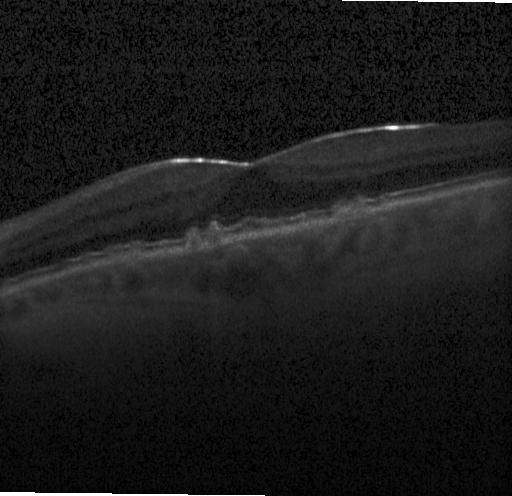

OCT line scan · spectral-domain OCT. Impression: multiple drusen.